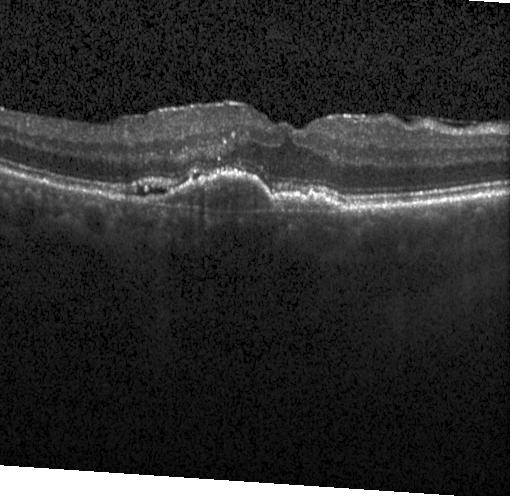
Impression: a choroidal neovascular membrane.